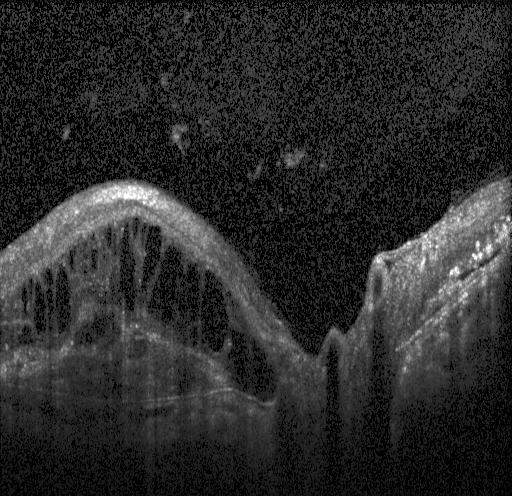 Optical coherence tomography scan; instrument: Heidelberg Spectralis; spectral-domain optical coherence tomography. Diagnosis: a choroidal neovascular membrane.